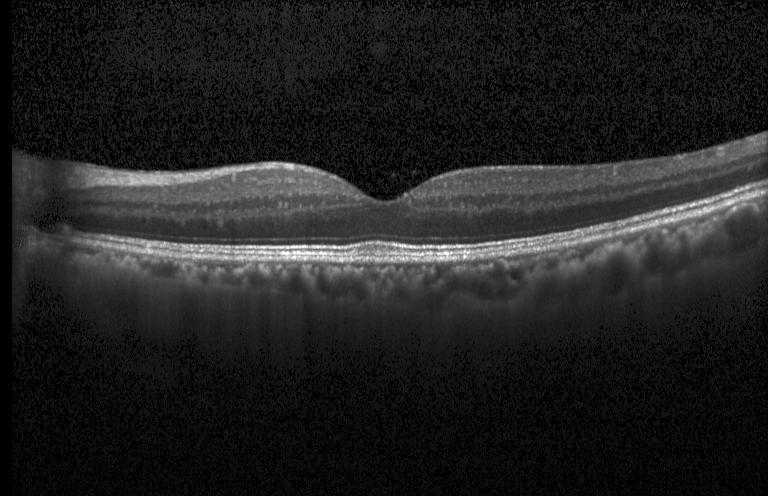
Retinal OCT B-scan. Impression: no choroidal neovascularization, diabetic macular edema, or drusen.